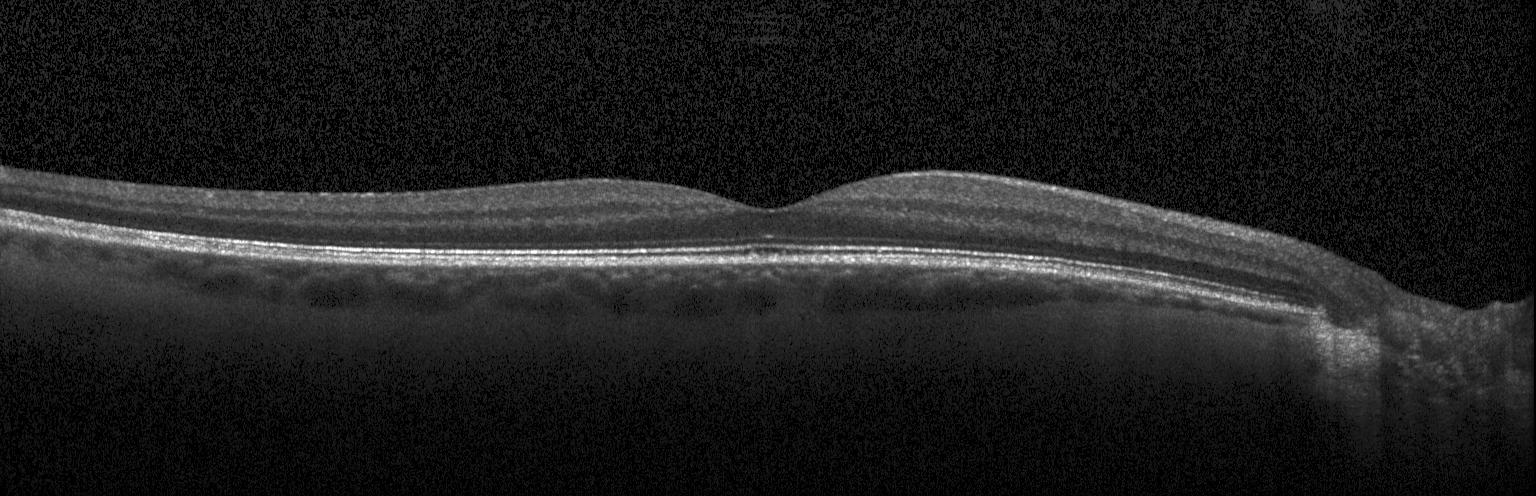
Through the macula; optical coherence tomography B-scan
OCT finding: no choroidal neovascularization, diabetic macular edema, or drusen.